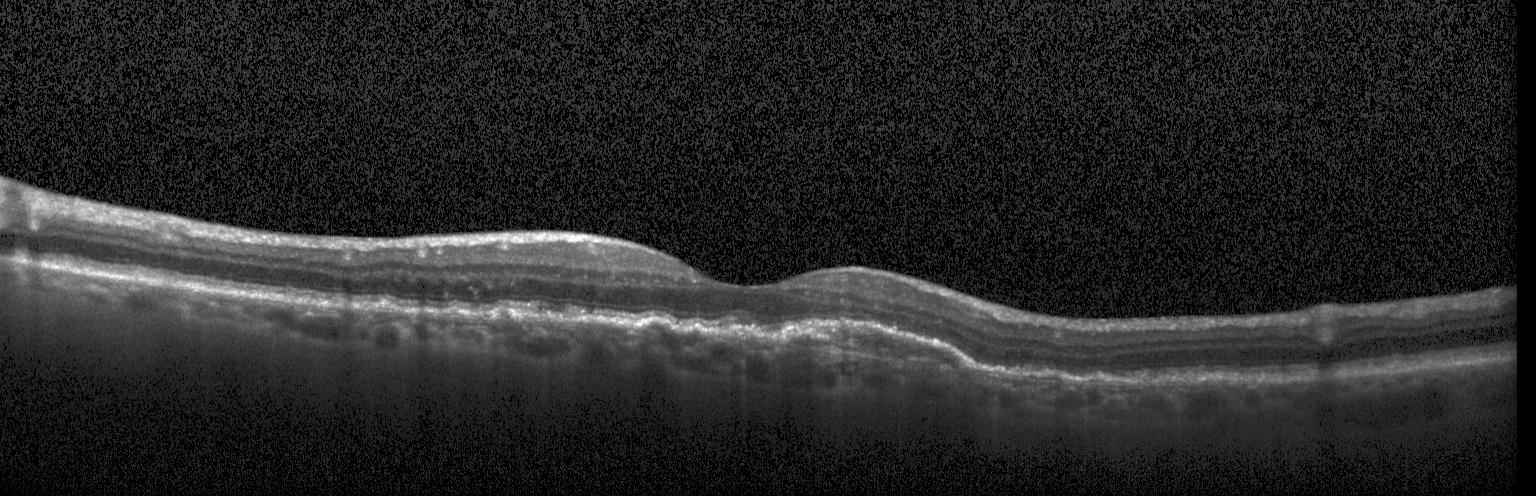

Horizontal scan through the fovea · optical coherence tomography scan · Heidelberg Spectralis OCT system.
OCT finding: a choroidal neovascular membrane.